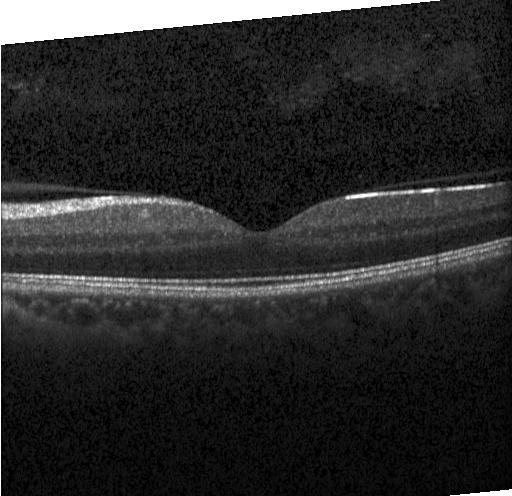 Retinal OCT cross-section showing no choroidal neovascularization, no diabetic macular edema, and no drusen.